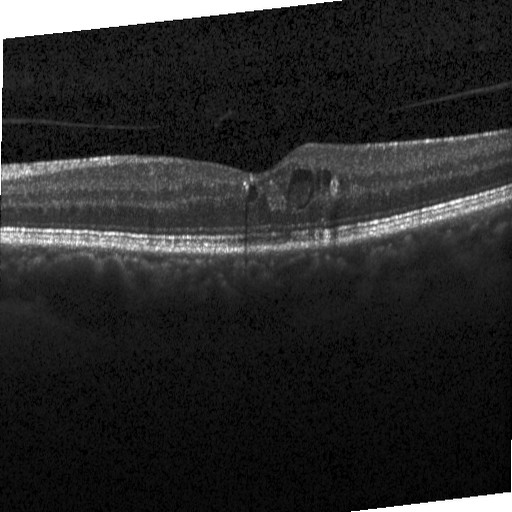 Diagnosis: diabetic macular edema.